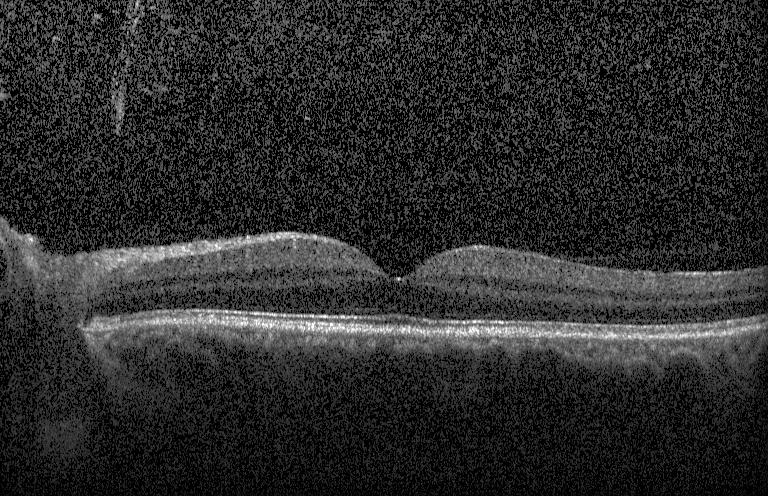

OCT B-scan · spectral-domain optical coherence tomography · centered on the fovea · Heidelberg Spectralis
No choroidal neovascularization, diabetic macular edema, or drusen.